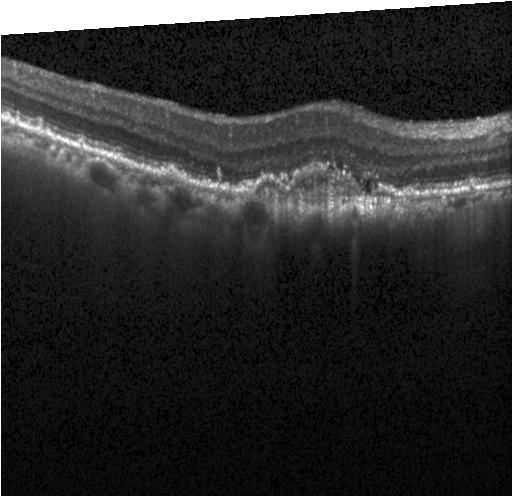 Retinal OCT B-scan.
A choroidal neovascular membrane.